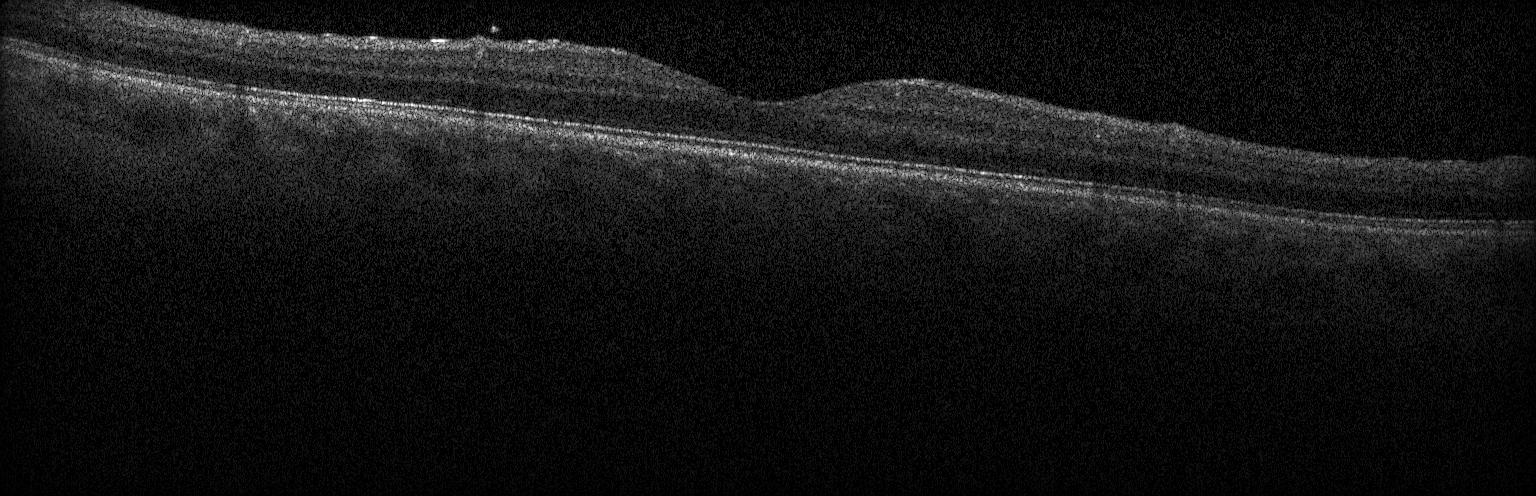 OCT B-scan
Finding: neither CNV, DME, nor drusen.